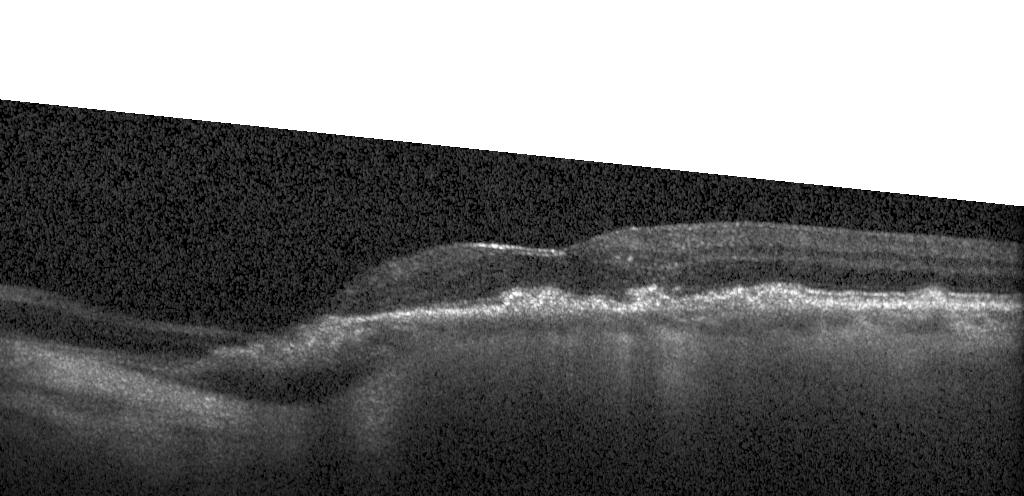
Retinal OCT cross-section. Instrument: Heidelberg Spectralis — Diagnosis: a choroidal neovascular membrane.